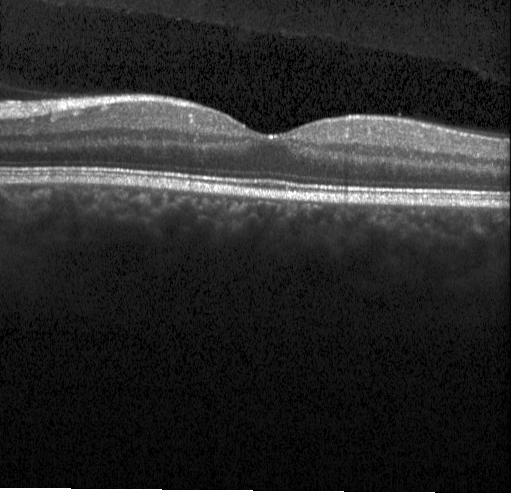
Heidelberg Spectralis; OCT B-scan.
The scan shows no evidence of CNV, DME, or drusen.